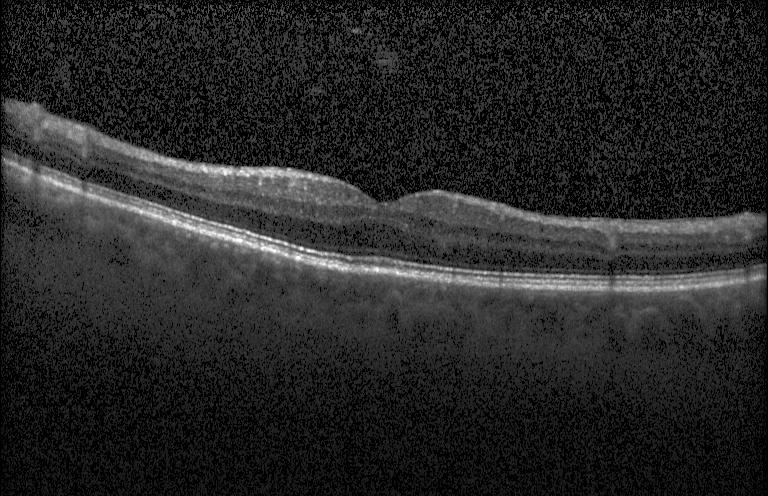 OCT B-scan showing no choroidal neovascularization, no diabetic macular edema, and no drusen.